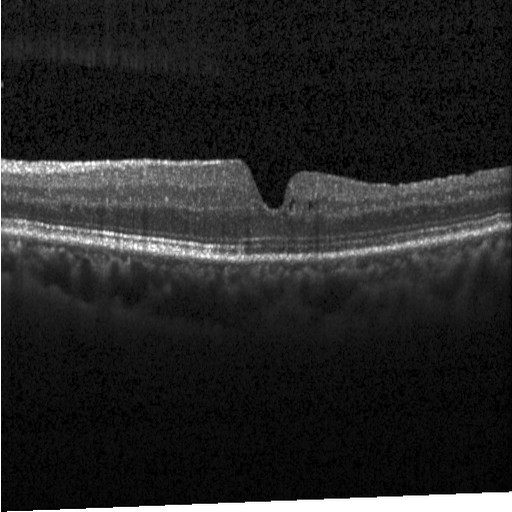

OCT scan showing diabetic macular edema (DME).